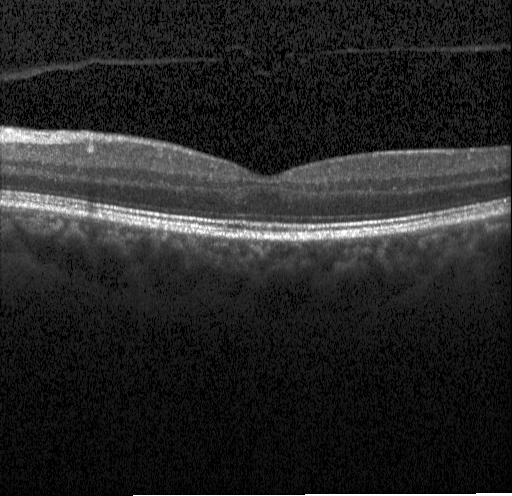

Heidelberg Spectralis. Optical coherence tomography B-scan. Through the macula. Assessment: no choroidal neovascularization, diabetic macular edema, or drusen.